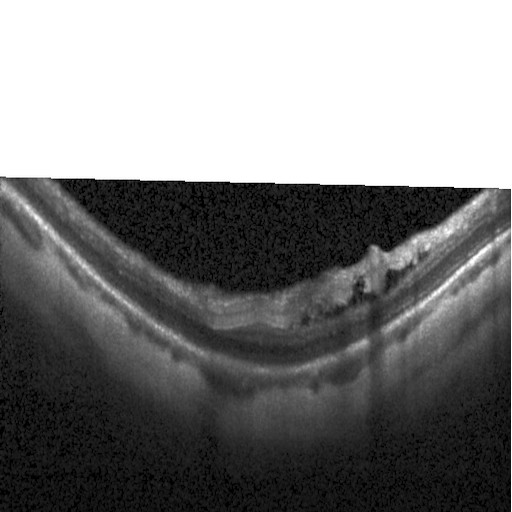 Centered on the fovea. Optical coherence tomography B-scan.
Diabetic macular edema.